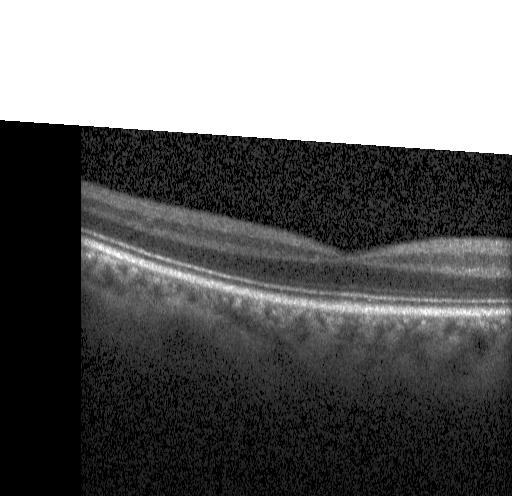
Finding: no evidence of CNV, DME, or drusen.